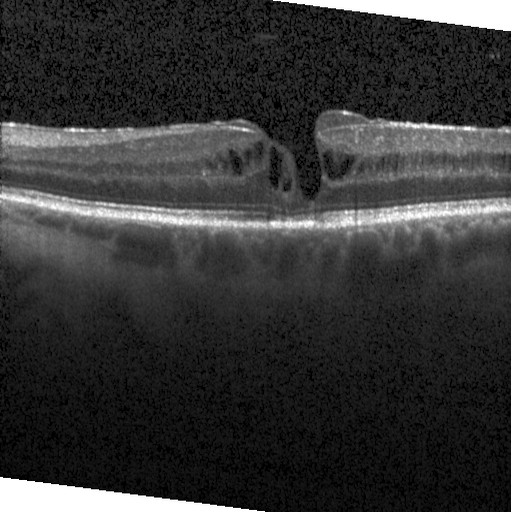 Heidelberg Spectralis · spectral-domain optical coherence tomography · optical coherence tomography B-scan. Finding: diabetic macular edema.